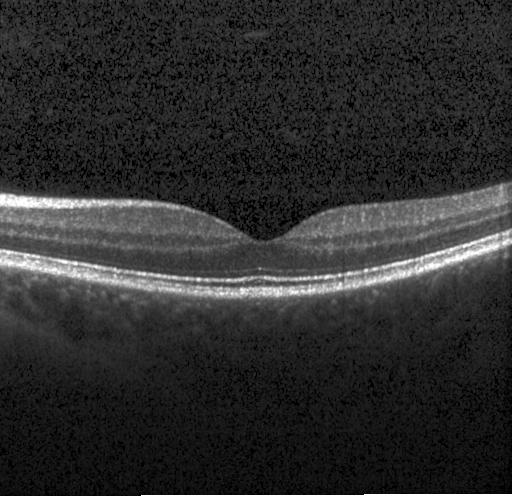
OCT B-scan showing no choroidal neovascularization, no diabetic macular edema, and no drusen.